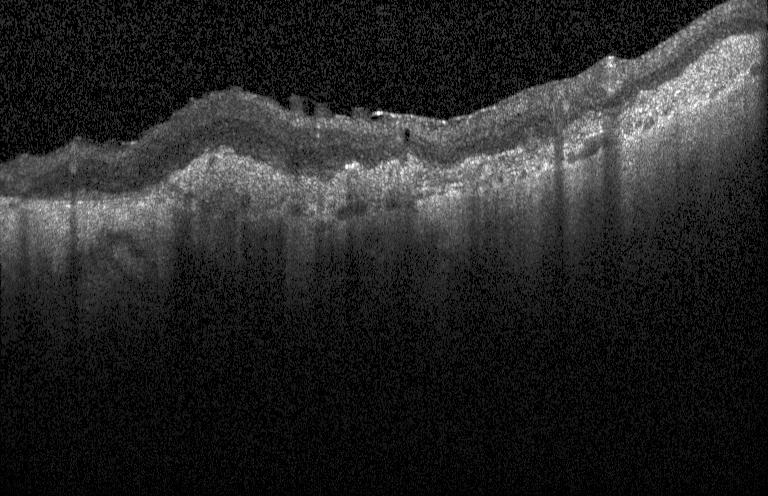
OCT line scan, spectral-domain OCT, macular scan
Finding: choroidal neovascularization (CNV).